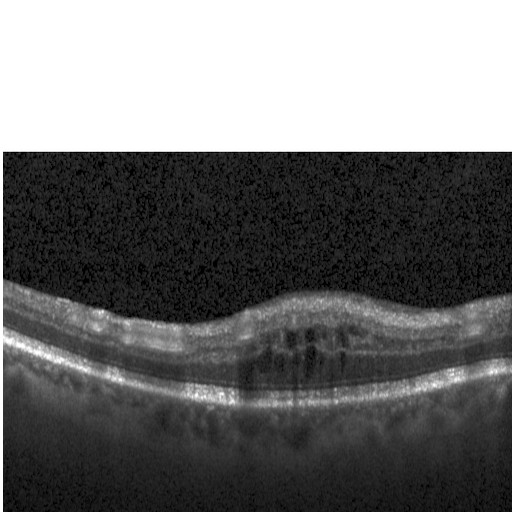
Impression: DME.